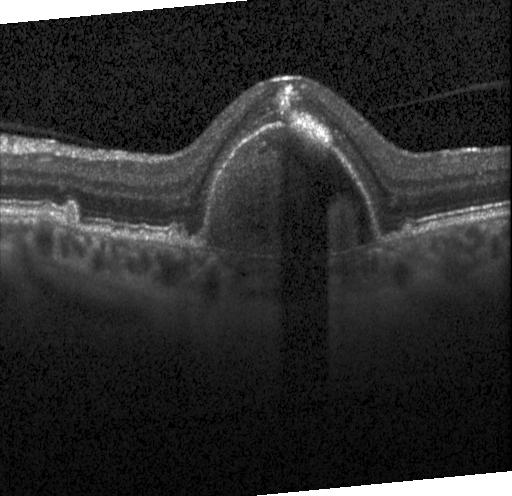

SD-OCT; OCT B-scan — The scan shows CNV.